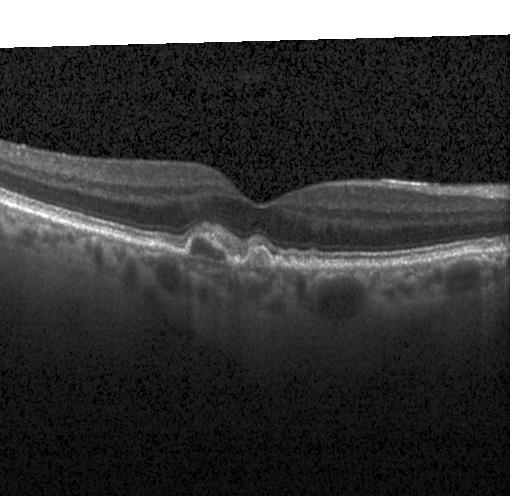 Centered on the fovea. Instrument: Heidelberg Spectralis. Retinal OCT B-scan. SD-OCT.
Impression: a choroidal neovascular membrane.